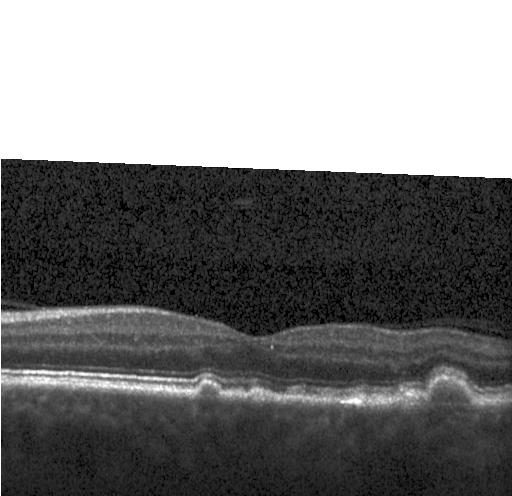
Horizontal scan through the fovea; SD-OCT; OCT line scan
Finding: drusen.